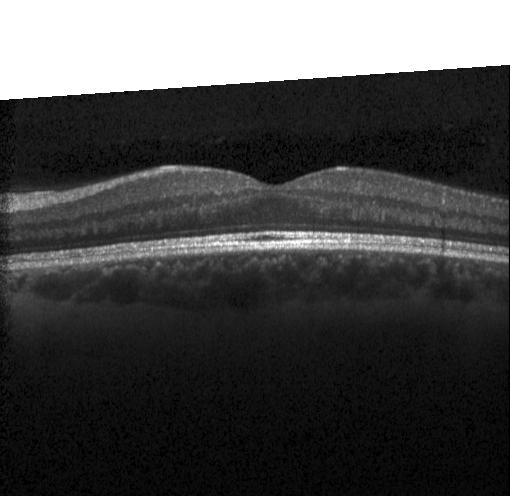
Instrument: Heidelberg Spectralis. Macular scan. Retinal OCT B-scan. The scan shows no choroidal neovascularization, diabetic macular edema, or drusen.